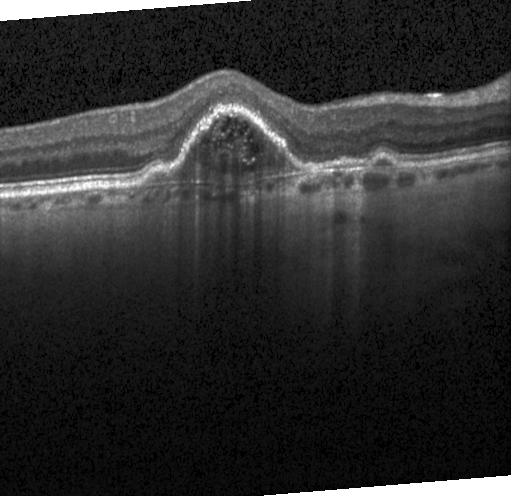
OCT scan showing choroidal neovascularization.